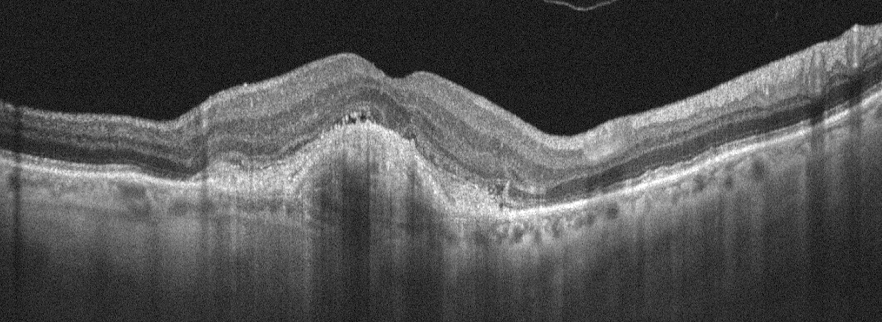 Oculus sinister · retinal OCT cross-section · Optovue Avanti RTVue XR · through the macula.
This B-scan demonstrates age-related macular degeneration (AMD).